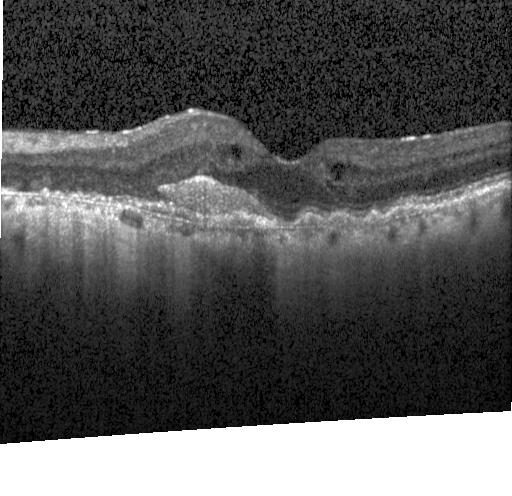 Retinal OCT cross-section. Finding: a choroidal neovascular membrane.